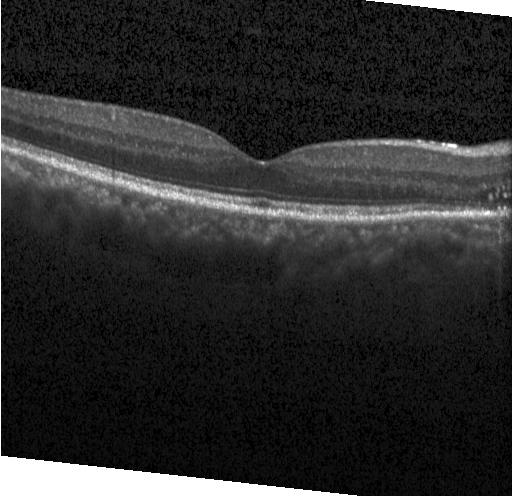 OCT finding: neither choroidal neovascularization, diabetic macular edema, nor drusen.